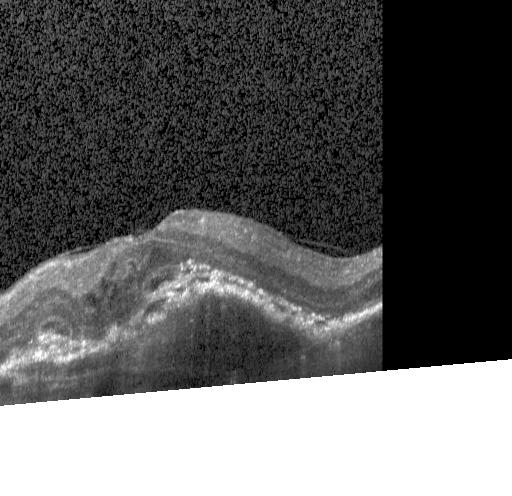 Spectral-domain OCT, instrument: Heidelberg Spectralis, OCT B-scan, horizontal scan through the fovea
OCT finding: CNV.